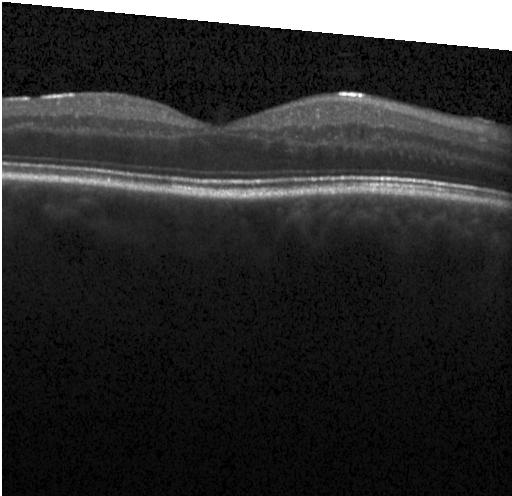 OCT line scan. Macular OCT: no CNV, DME, or drusen.